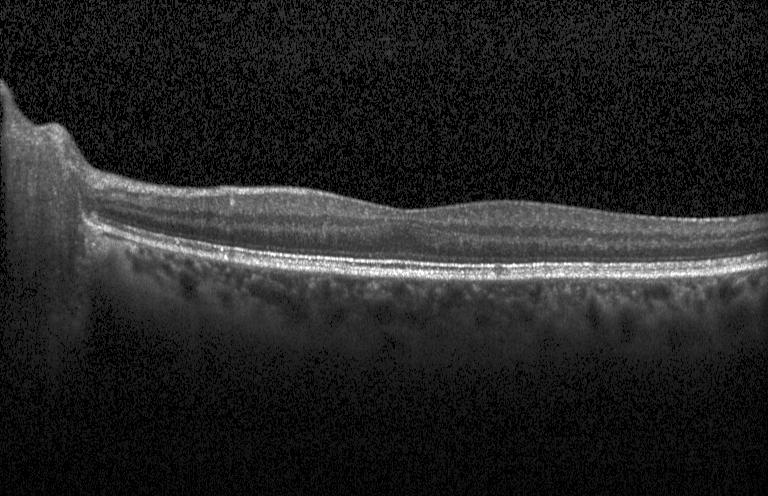 OCT B-scan — No CNV, DME, or drusen.